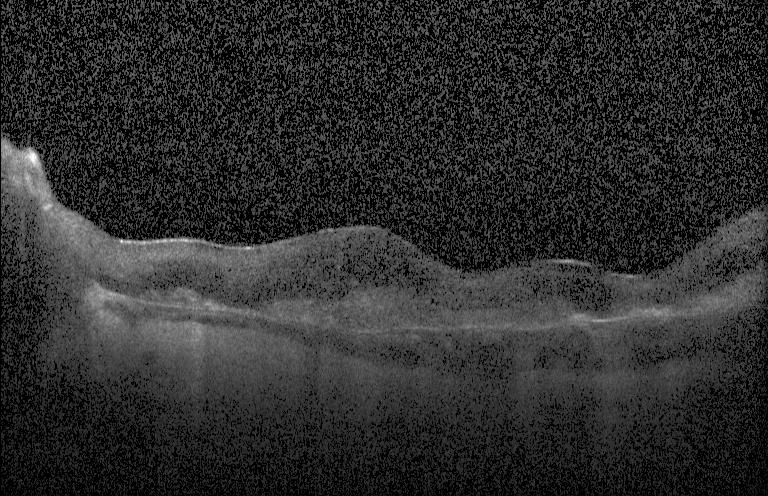
Macular scan · optical coherence tomography scan. Macular OCT: a choroidal neovascular membrane.